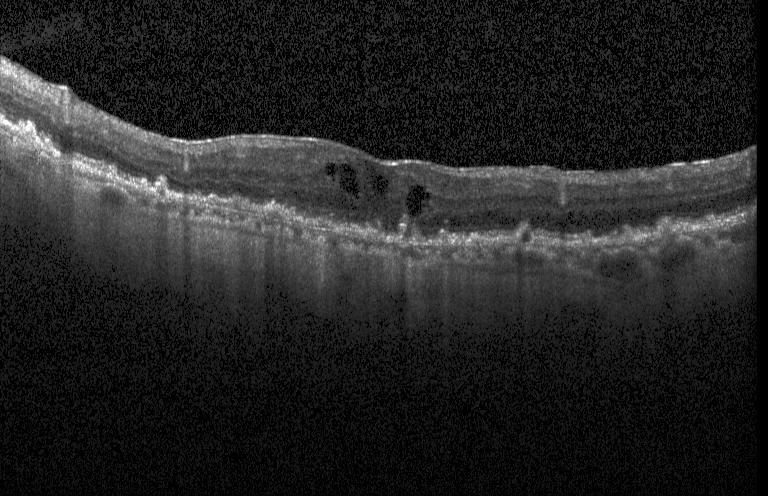
Through the macula · SD-OCT · OCT line scan · acquired on a Heidelberg Spectralis.
OCT finding: choroidal neovascularization.